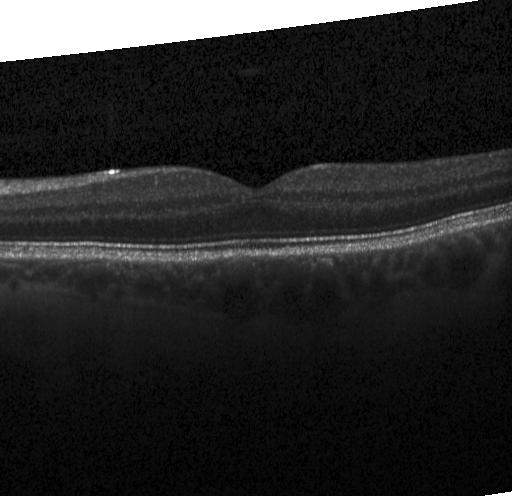
OCT scan showing no choroidal neovascularization, no diabetic macular edema, and no drusen.